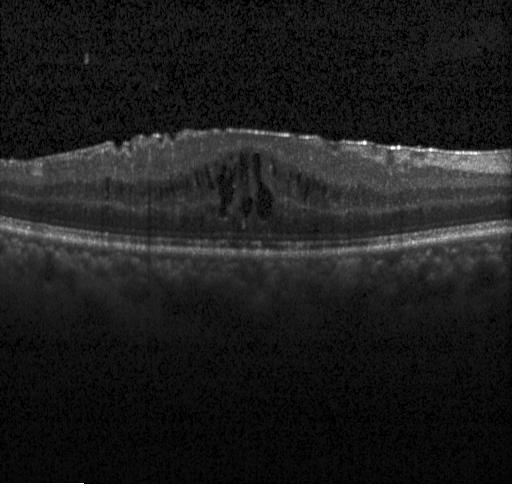
Spectral-domain OCT; retinal OCT cross-section; horizontal scan through the fovea — Finding: diabetic macular edema (DME).